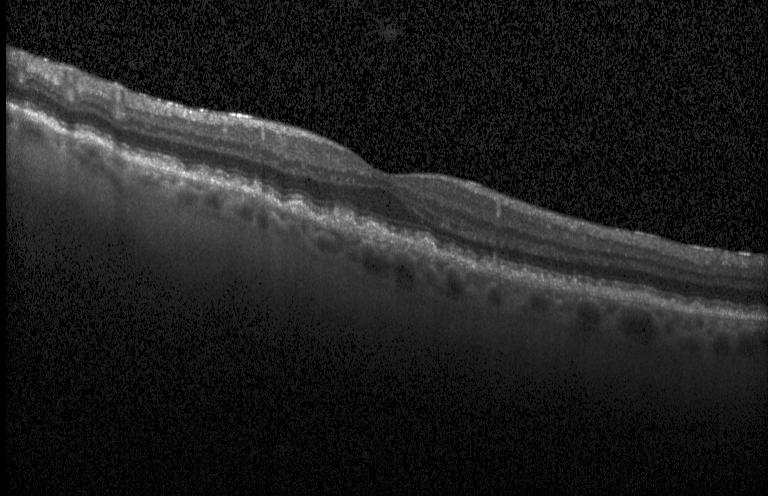

Assessment: sub-RPE drusenoid deposits.